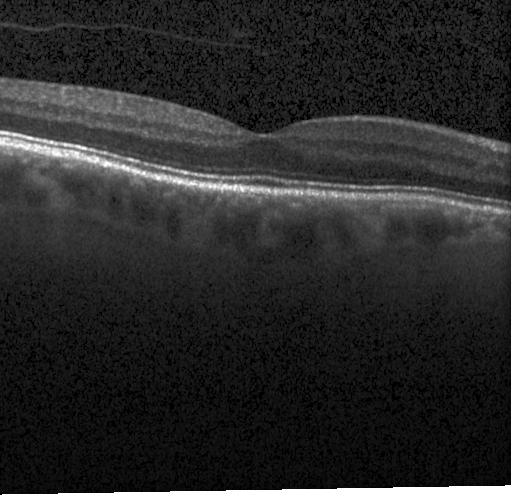 Dx: neither choroidal neovascularization, diabetic macular edema, nor drusen.